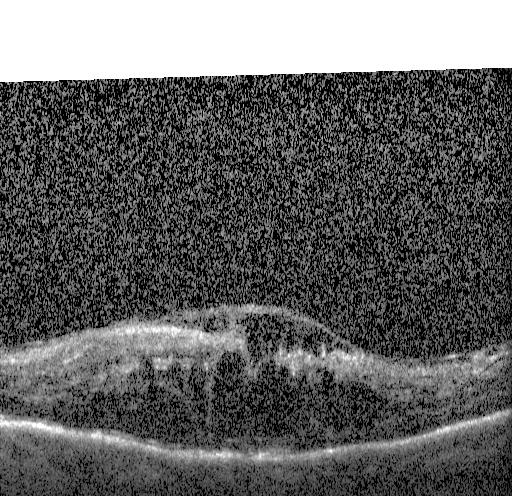
Retinal OCT cross-section — Finding: diabetic macular edema (DME).